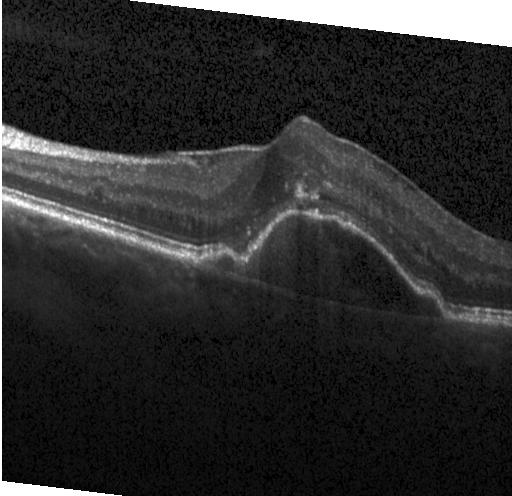

Spectral-domain optical coherence tomography; Heidelberg Spectralis; fovea-centered; retinal OCT B-scan — This B-scan demonstrates choroidal neovascularization.